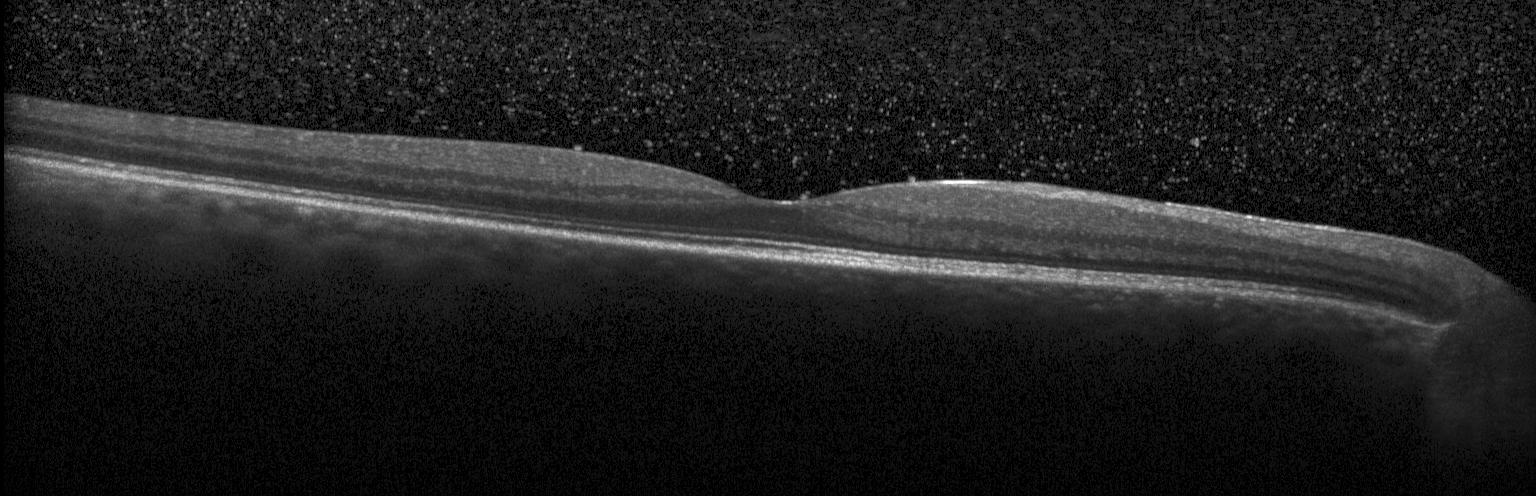

Macular OCT demonstrating no choroidal neovascularization, no diabetic macular edema, and no drusen.